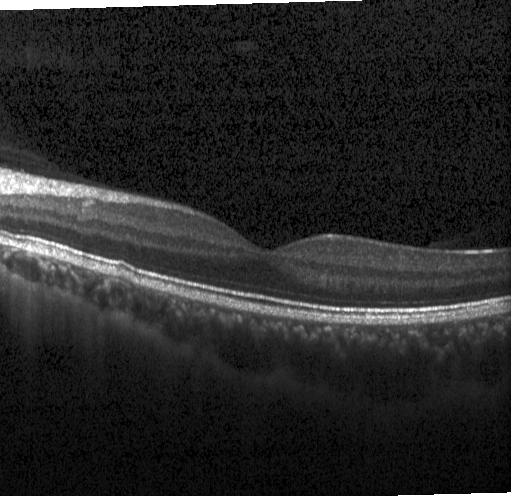 Finding: sub-RPE drusenoid deposits.